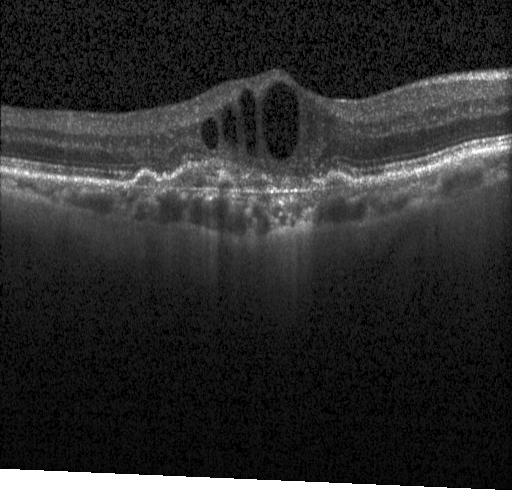

Retinal OCT cross-section
Diagnosis: choroidal neovascularization.